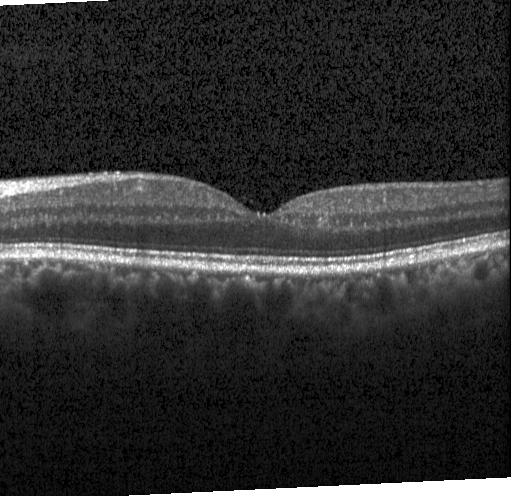
Neither choroidal neovascularization, diabetic macular edema, nor drusen.